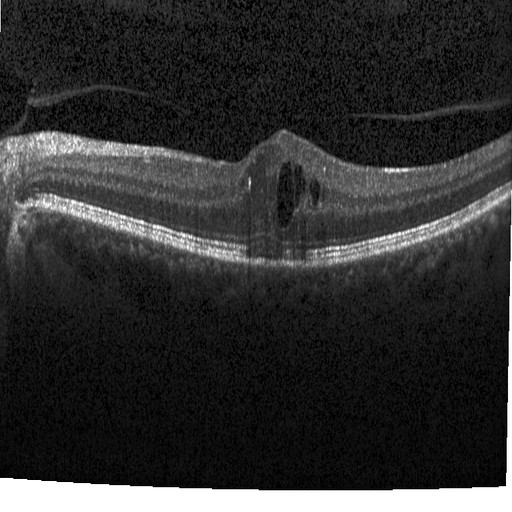
Spectral-domain OCT B-scan: DME.